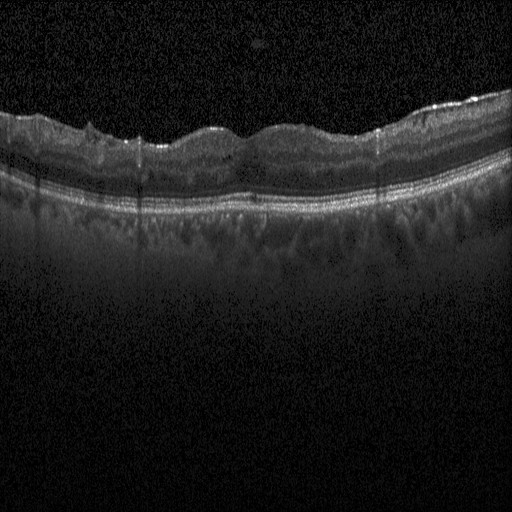 Impression: DME.